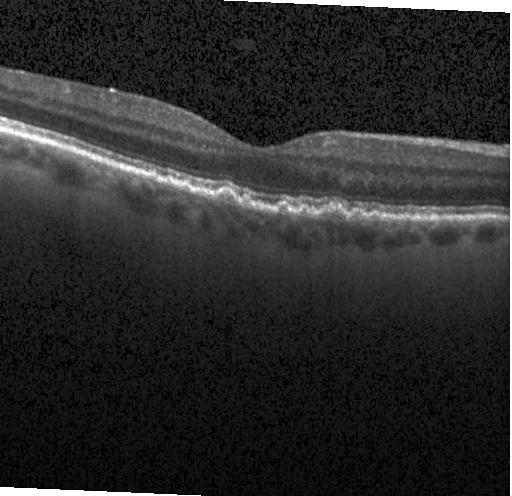
Spectral-domain optical coherence tomography. Fovea-centered. OCT B-scan
Finding: multiple drusen.